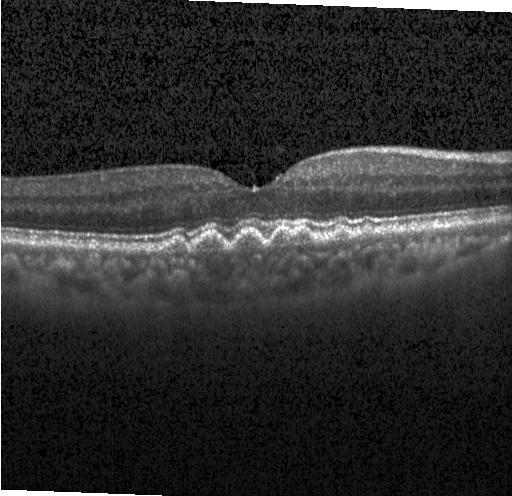

Optical coherence tomography B-scan, Heidelberg Spectralis OCT system
Finding: sub-RPE drusenoid deposits.